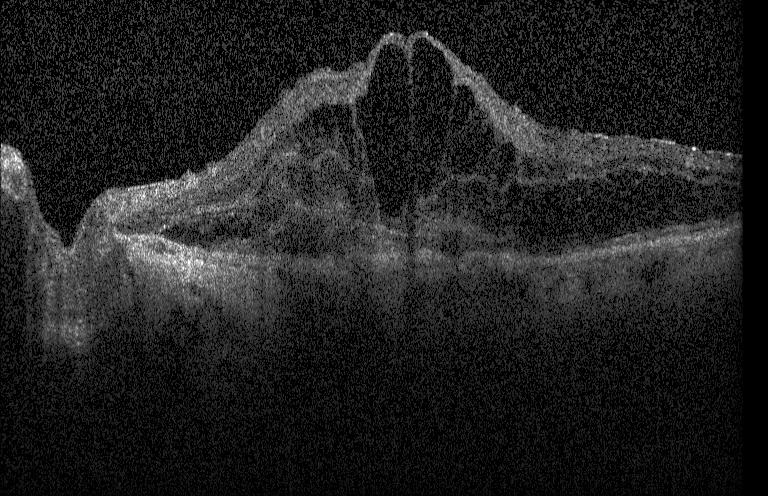

Acquired on a Heidelberg Spectralis. Optical coherence tomography scan. Spectral-domain OCT. Diagnosis: choroidal neovascularization (CNV).